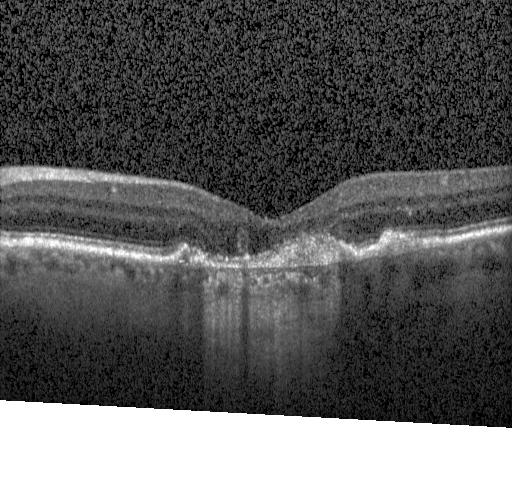 Fovea-centered; spectral-domain OCT; retinal OCT cross-section — Dx: CNV.